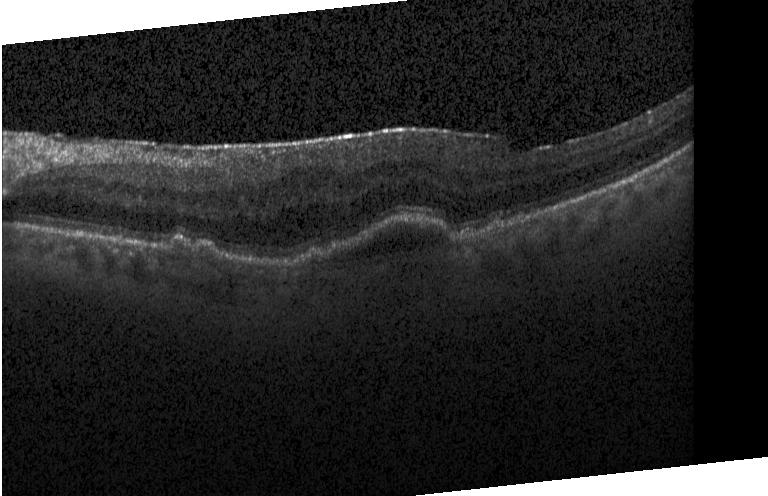
Centered on the fovea, OCT line scan, Heidelberg Spectralis OCT system — CNV.